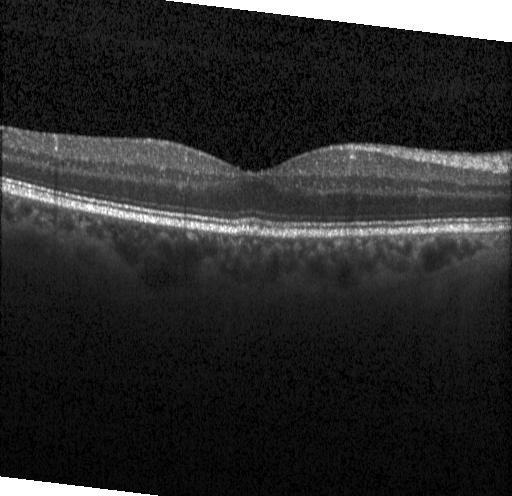
Spectral-domain OCT · optical coherence tomography scan · macular scan · Heidelberg Spectralis OCT system. Diagnosis: no evidence of CNV, DME, or drusen.